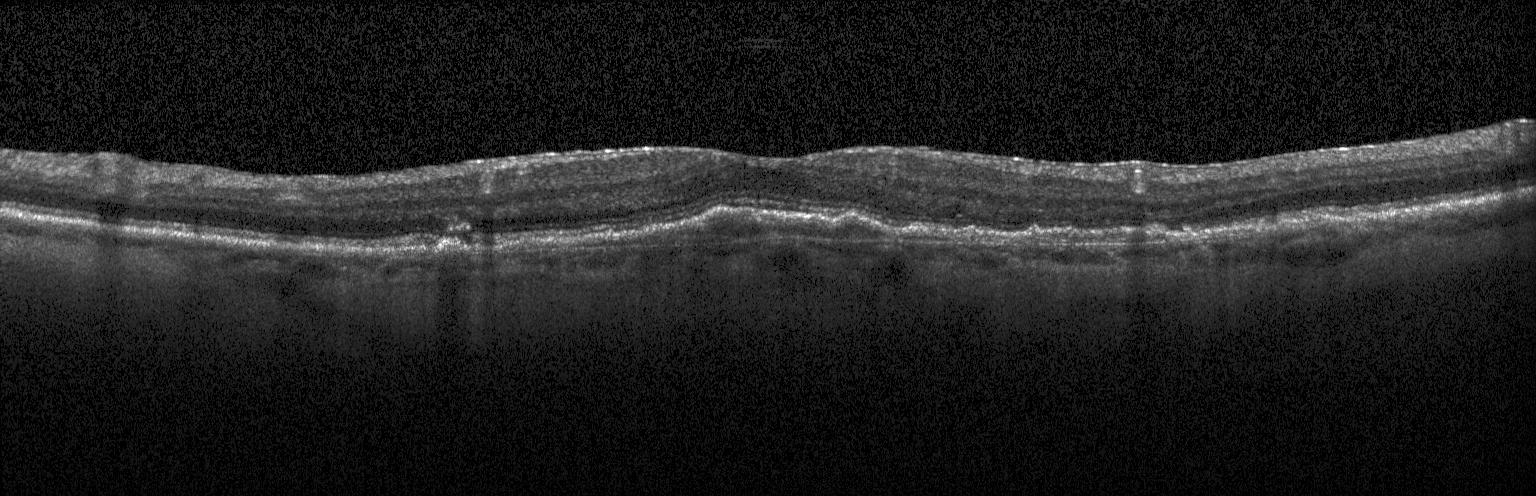

Retinal OCT B-scan — A choroidal neovascular membrane.